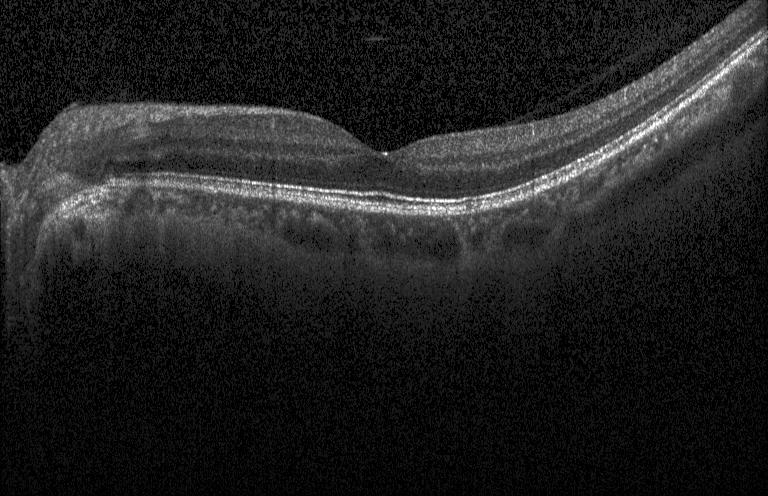 Optical coherence tomography B-scan. Spectral-domain OCT. Heidelberg Spectralis. Fovea-centered — This B-scan demonstrates no choroidal neovascularization, no diabetic macular edema, and no drusen.